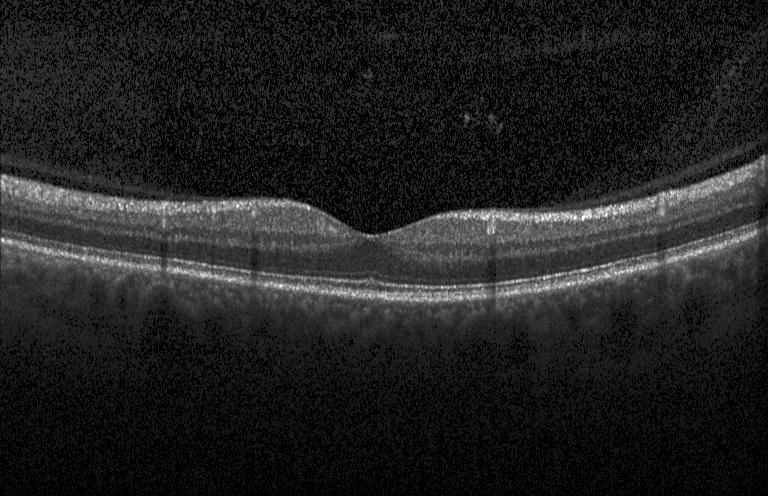 Diagnosis: no evidence of choroidal neovascularization, diabetic macular edema, or drusen.